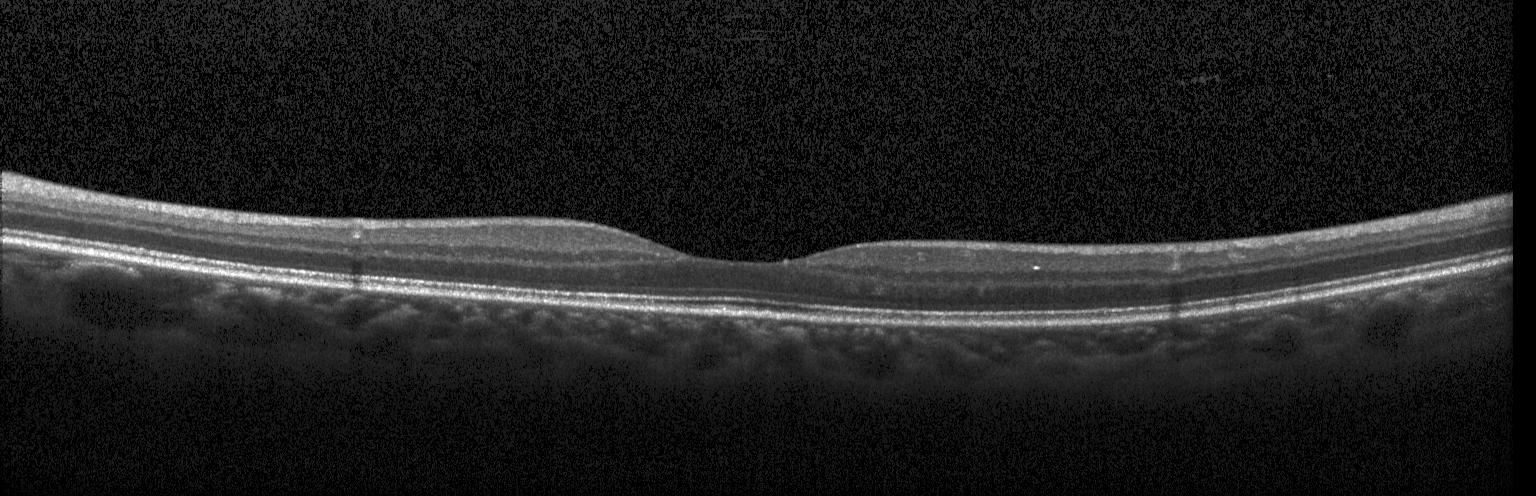

SD-OCT · Heidelberg Spectralis OCT system · retinal OCT cross-section · through the macula. Assessment: neither choroidal neovascularization, diabetic macular edema, nor drusen.